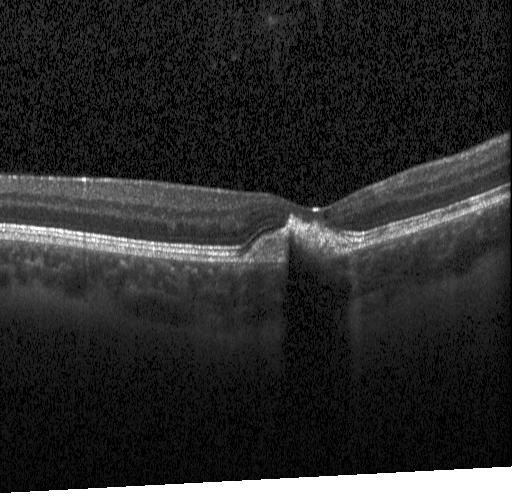
Optical coherence tomography B-scan; instrument: Heidelberg Spectralis; macular scan
The scan shows choroidal neovascularization.